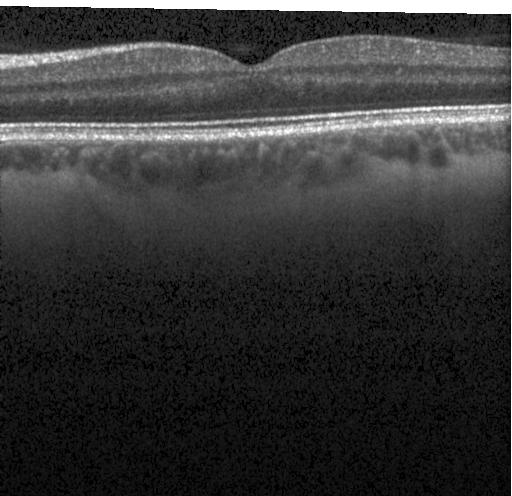 SD-OCT, fovea-centered, retinal OCT B-scan, Heidelberg Spectralis — The scan shows neither CNV, DME, nor drusen.